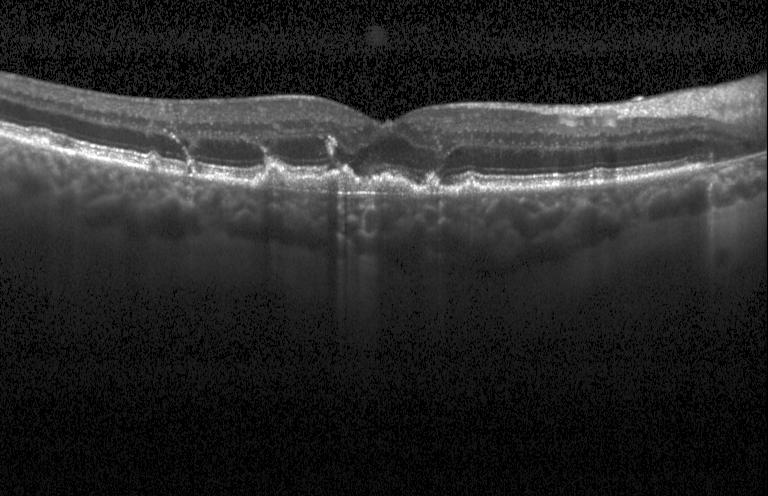

OCT B-scan · acquired on a Heidelberg Spectralis · SD-OCT
Finding: CNV.